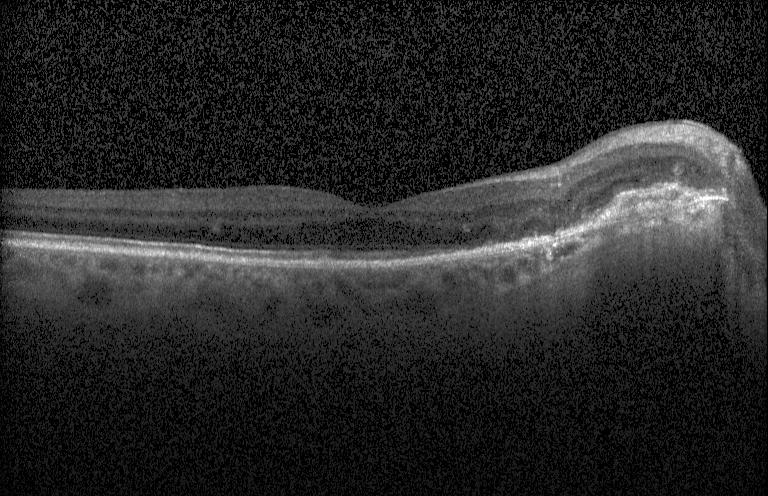
Retinal OCT B-scan. Macular scan. Spectral-domain OCT. Heidelberg Spectralis. Macular OCT: a choroidal neovascular membrane.